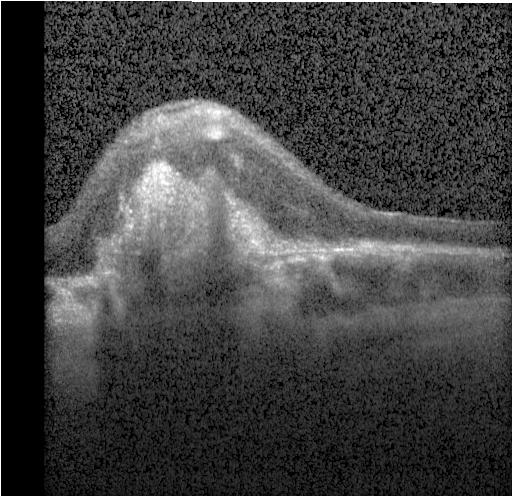 Instrument: Heidelberg Spectralis. Spectral-domain OCT. Fovea-centered. Retinal OCT B-scan.
This B-scan demonstrates CNV.